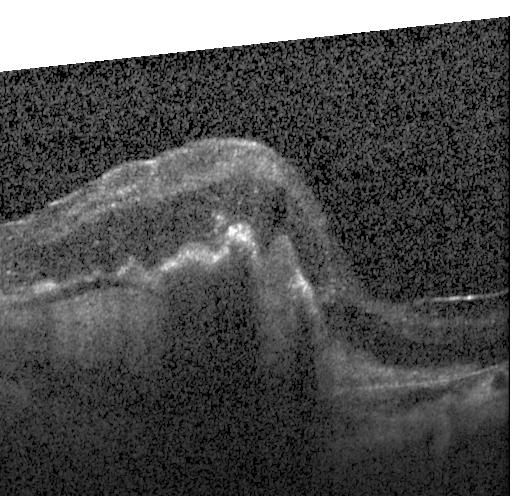

Retinal OCT cross-section
A choroidal neovascular membrane.